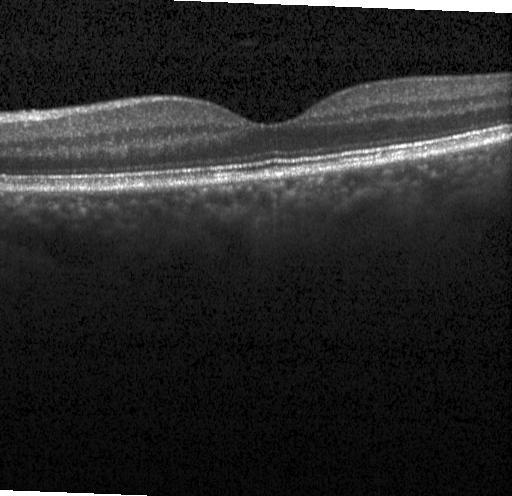

Heidelberg Spectralis; spectral-domain optical coherence tomography; horizontal scan through the fovea; optical coherence tomography scan. No evidence of choroidal neovascularization, diabetic macular edema, or drusen.